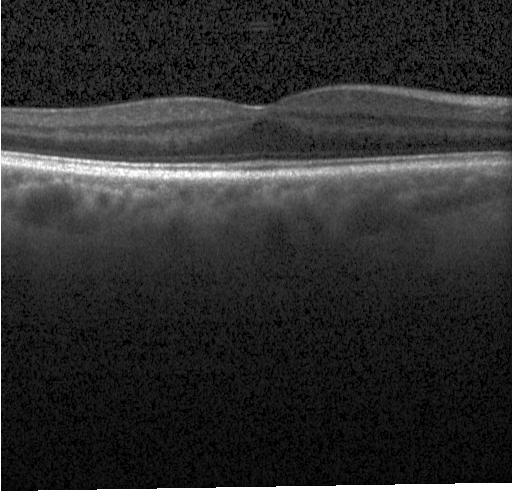
Impression: no choroidal neovascularization, no diabetic macular edema, and no drusen.